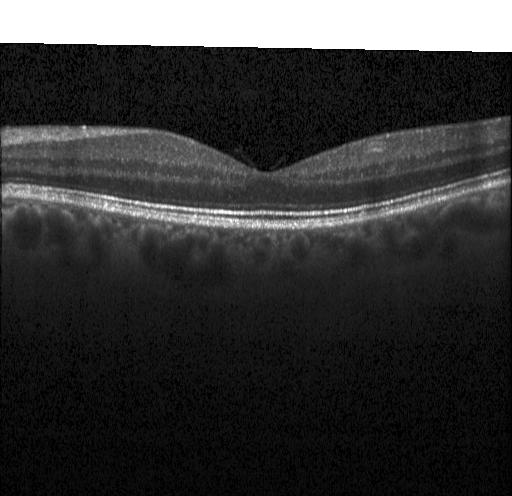
This B-scan demonstrates no choroidal neovascularization, diabetic macular edema, or drusen.